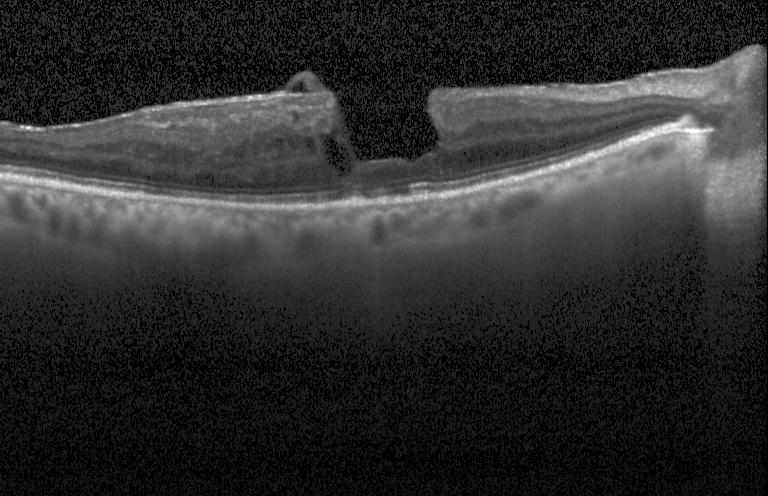 Macular OCT: diabetic macular edema.